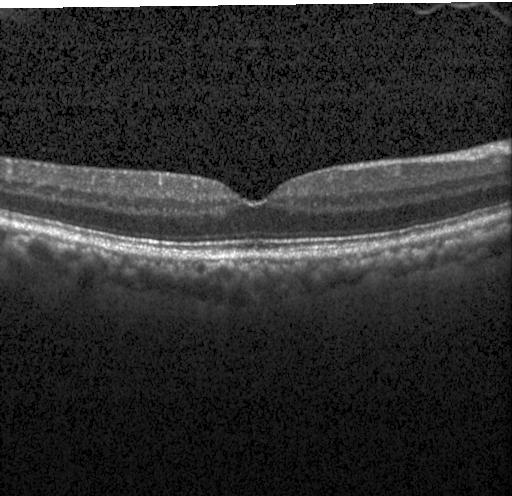
OCT finding: neither choroidal neovascularization, diabetic macular edema, nor drusen.